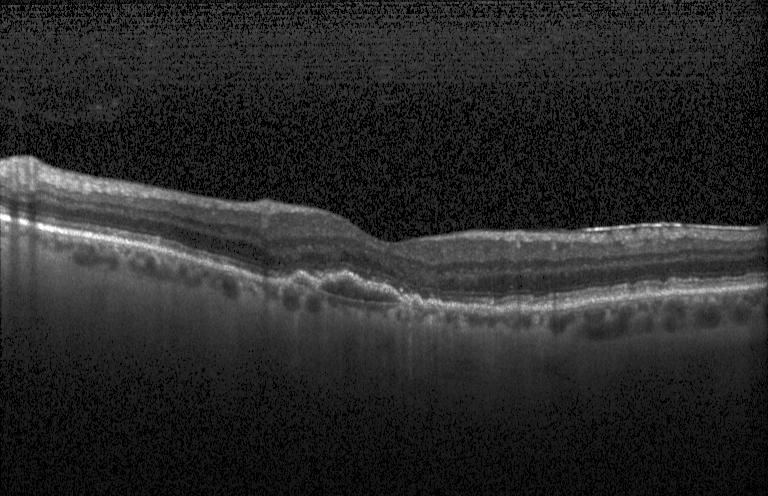

Optical coherence tomography B-scan — Impression: a choroidal neovascular membrane.